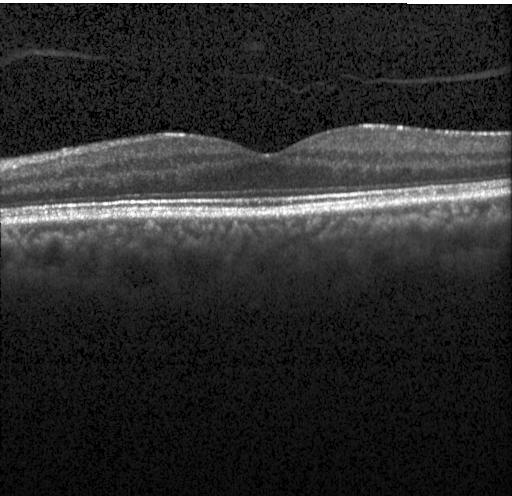 OCT scan showing no choroidal neovascularization, diabetic macular edema, or drusen.